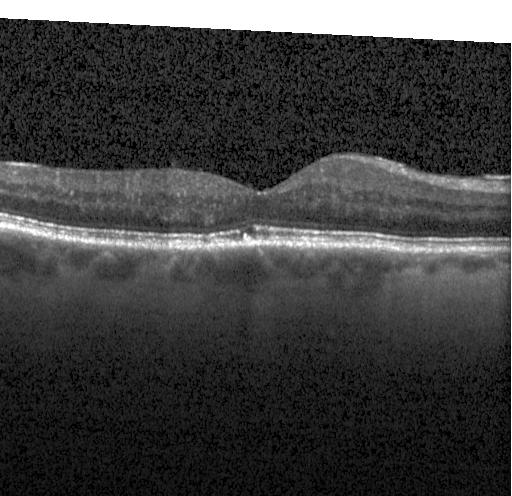

Spectral-domain OCT B-scan: multiple drusen.